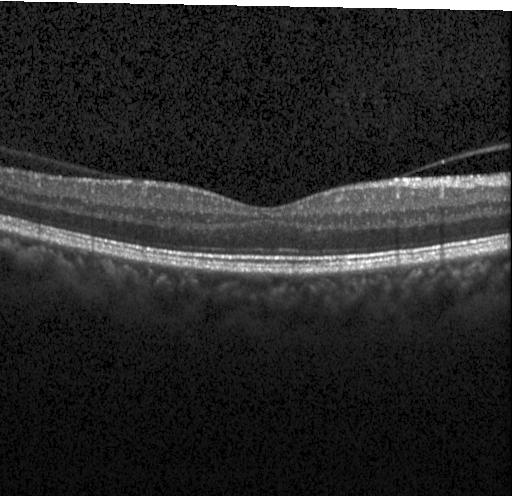
Optical coherence tomography B-scan — Finding: no choroidal neovascularization, no diabetic macular edema, and no drusen.